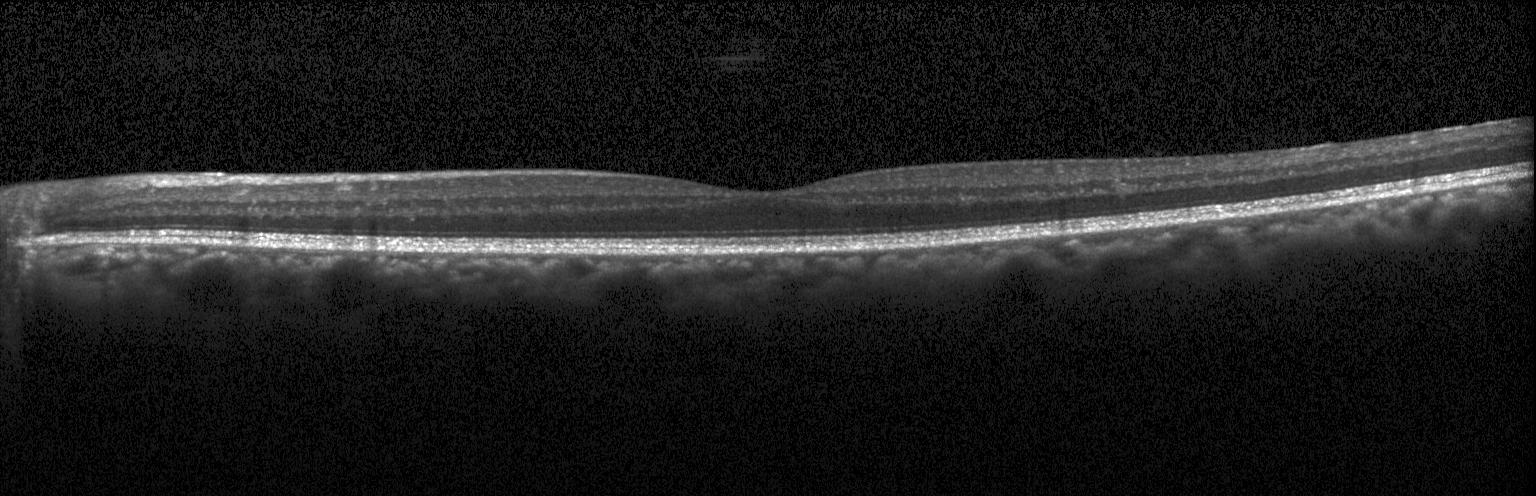

Impression: neither choroidal neovascularization, diabetic macular edema, nor drusen.